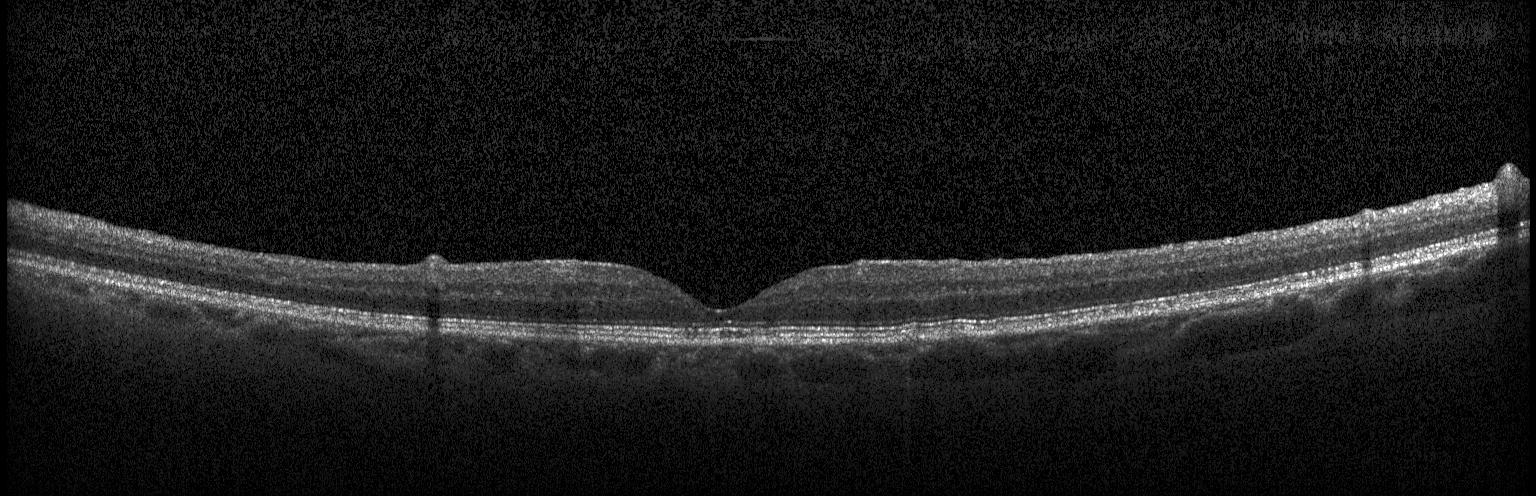 Horizontal scan through the fovea; spectral-domain optical coherence tomography; acquired on a Heidelberg Spectralis; OCT line scan.
Assessment: neither CNV, DME, nor drusen.